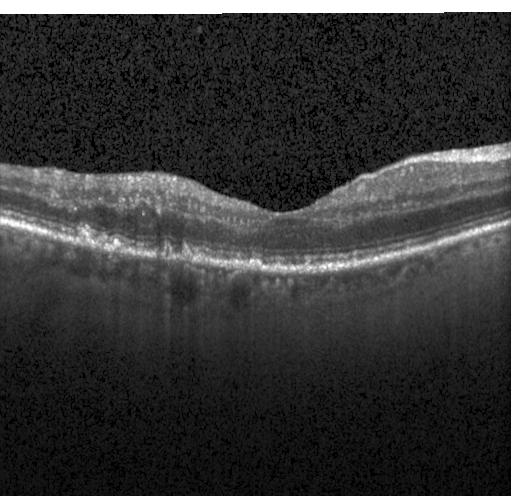
Optical coherence tomography scan · macular scan · Heidelberg Spectralis
Macular OCT: drusen.